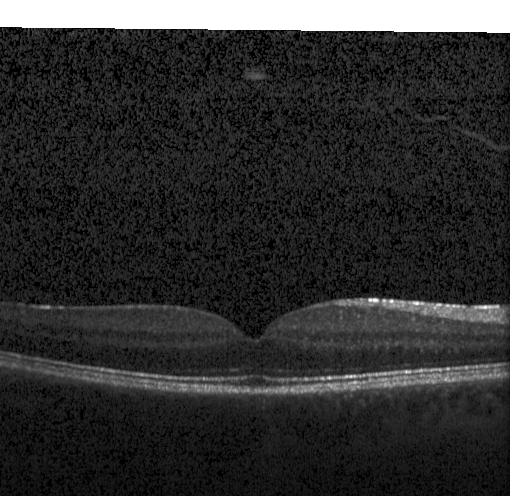

OCT B-scan
Diagnosis: neither choroidal neovascularization, diabetic macular edema, nor drusen.